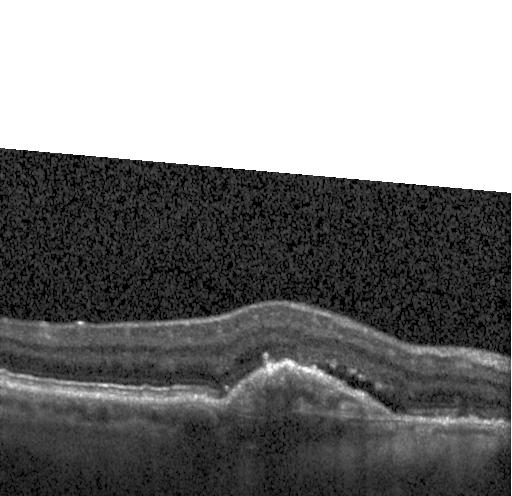
Macular OCT: choroidal neovascularization (CNV).